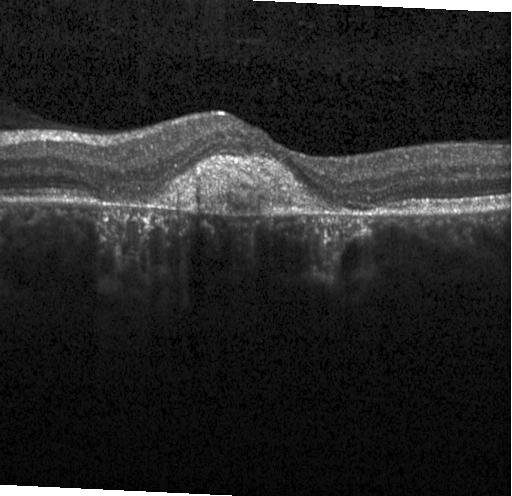

Impression: choroidal neovascularization.